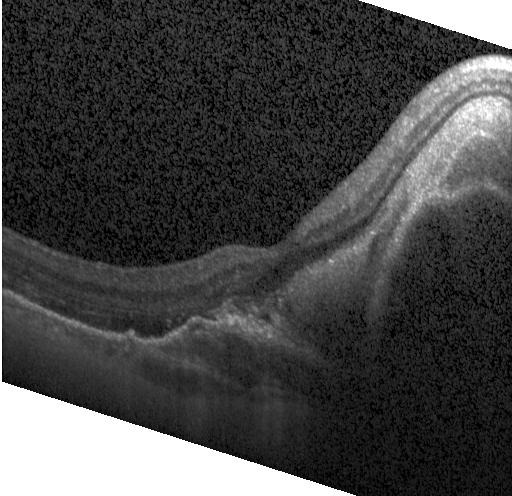 Spectral-domain OCT B-scan: CNV.